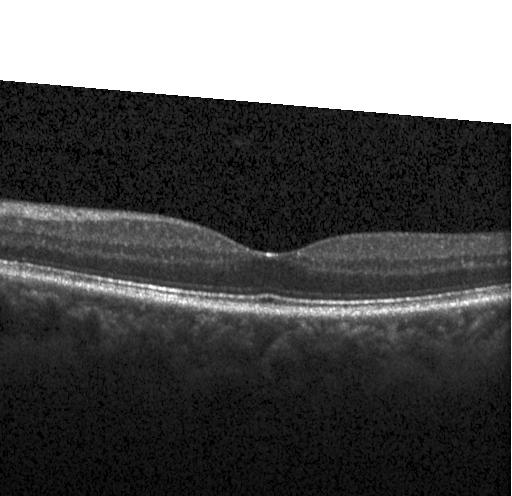
Instrument: Heidelberg Spectralis · optical coherence tomography scan — No evidence of choroidal neovascularization, diabetic macular edema, or drusen.